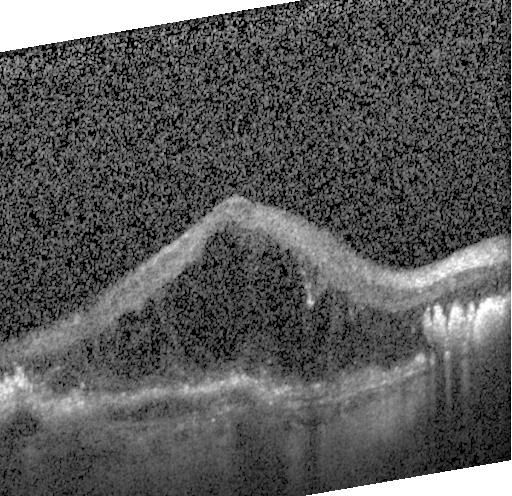

Finding: choroidal neovascularization.